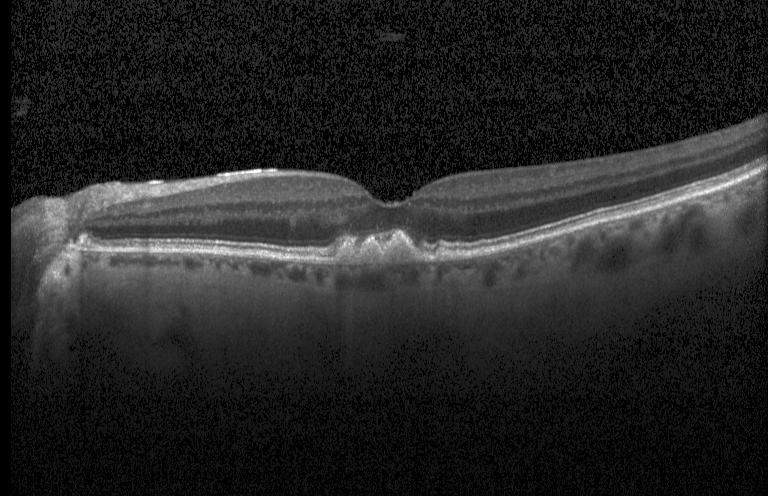 Spectral-domain OCT · retinal OCT B-scan
This B-scan demonstrates sub-RPE drusenoid deposits.